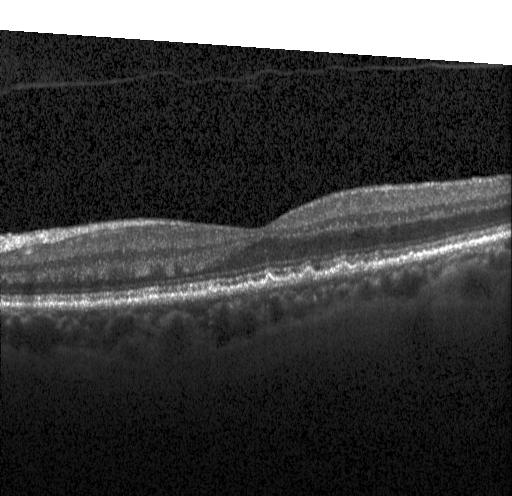
Optical coherence tomography scan, fovea-centered, spectral-domain optical coherence tomography — Finding: drusen.